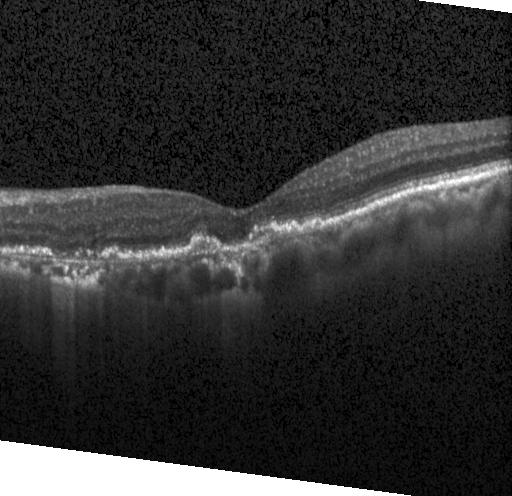 OCT B-scan; Heidelberg Spectralis; SD-OCT; horizontal scan through the fovea — Finding: a choroidal neovascular membrane.